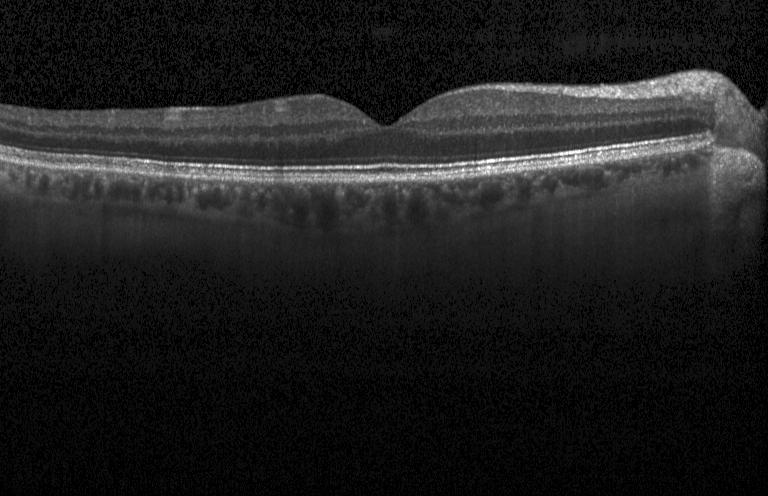 Optical coherence tomography scan — This B-scan demonstrates no choroidal neovascularization, diabetic macular edema, or drusen.